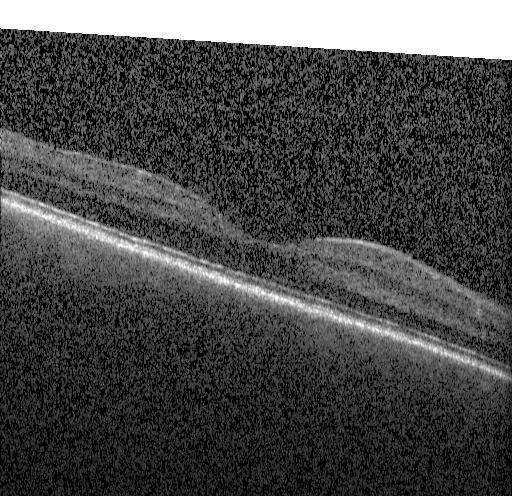

Instrument: Heidelberg Spectralis · spectral-domain OCT · centered on the fovea · retinal OCT cross-section. Diagnosis: no choroidal neovascularization, no diabetic macular edema, and no drusen.